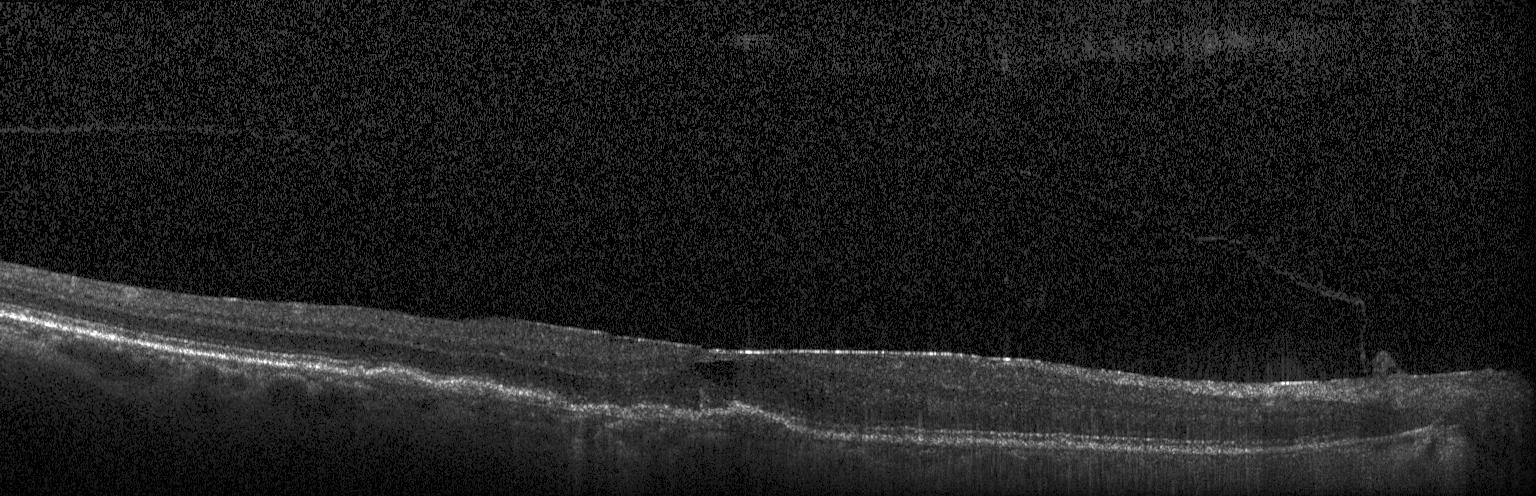
Impression: a choroidal neovascular membrane.